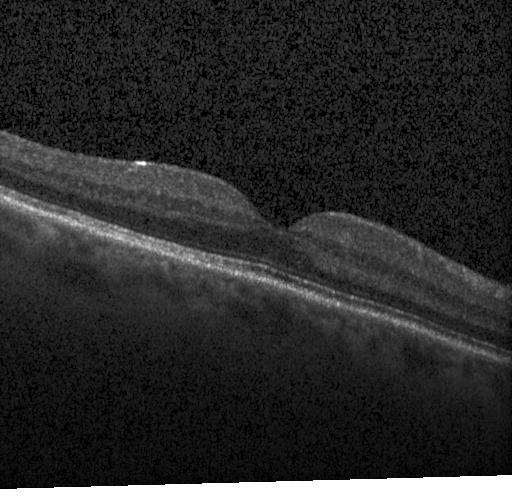

Optical coherence tomography B-scan, horizontal scan through the fovea. Diagnosis: no evidence of choroidal neovascularization, diabetic macular edema, or drusen.